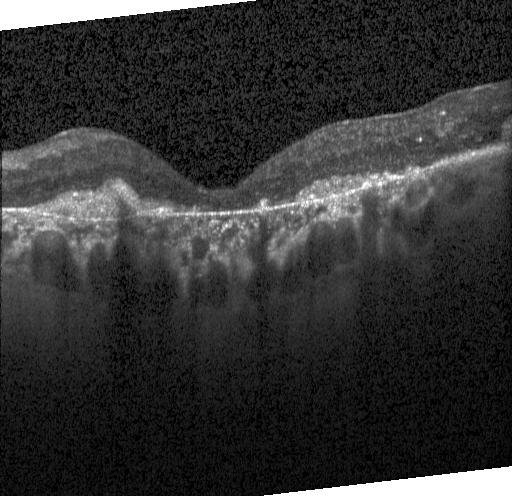
Retinal OCT cross-section
Diagnosis: CNV.